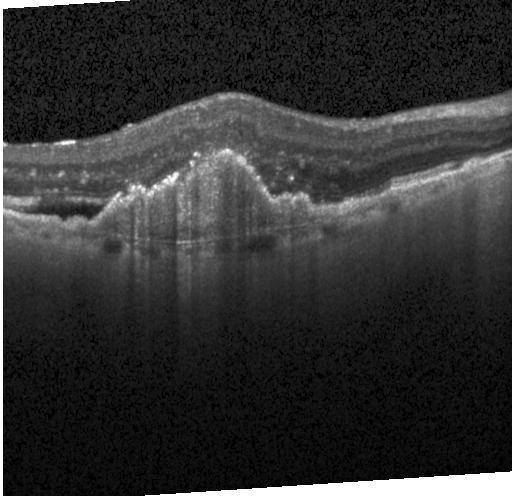
Spectral-domain OCT · Heidelberg Spectralis · retinal OCT B-scan.
Diagnosis: a choroidal neovascular membrane.